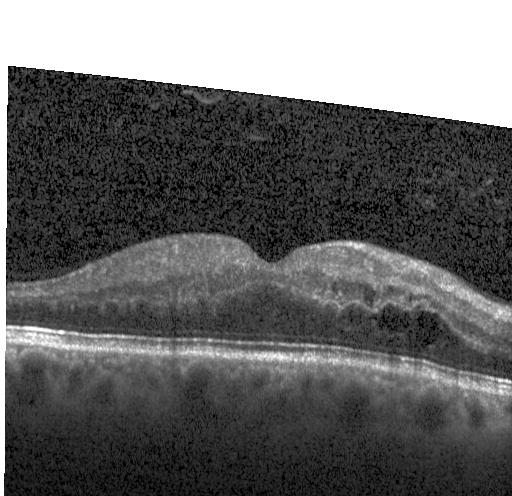 Optical coherence tomography B-scan · spectral-domain OCT · macular scan · Heidelberg Spectralis. OCT finding: diabetic macular edema (DME).